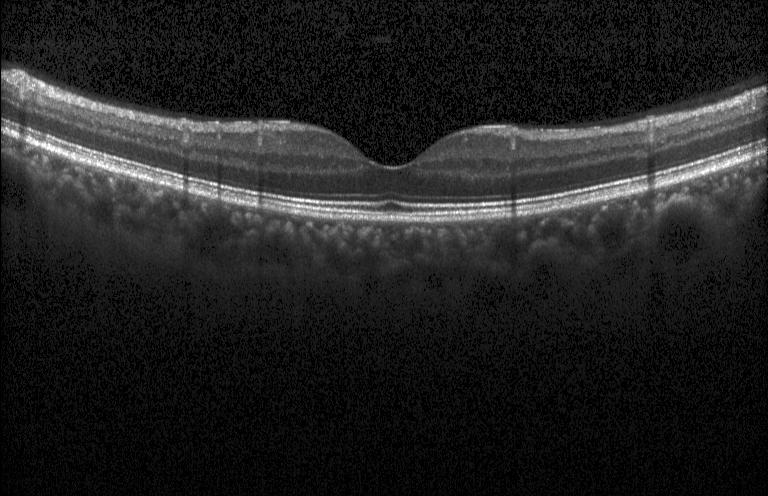 Impression: no choroidal neovascularization, diabetic macular edema, or drusen.